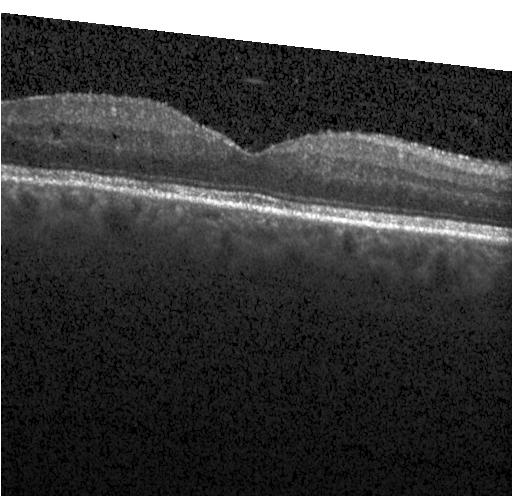

Spectral-domain OCT B-scan: no evidence of choroidal neovascularization, diabetic macular edema, or drusen.